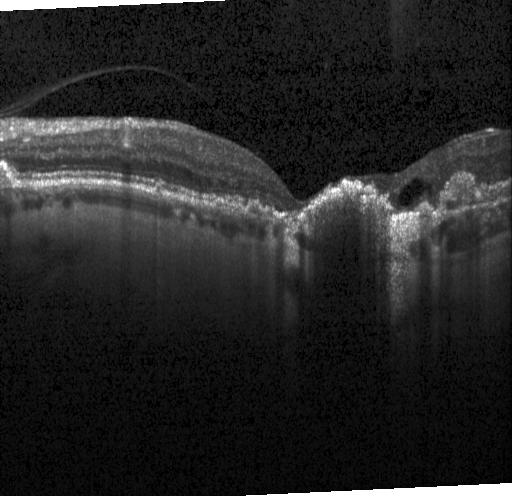
Centered on the fovea, retinal OCT cross-section
The scan shows a choroidal neovascular membrane.